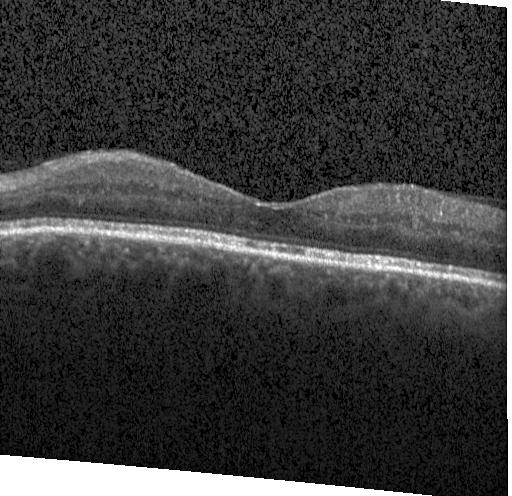
OCT B-scan. Finding: no evidence of CNV, DME, or drusen.